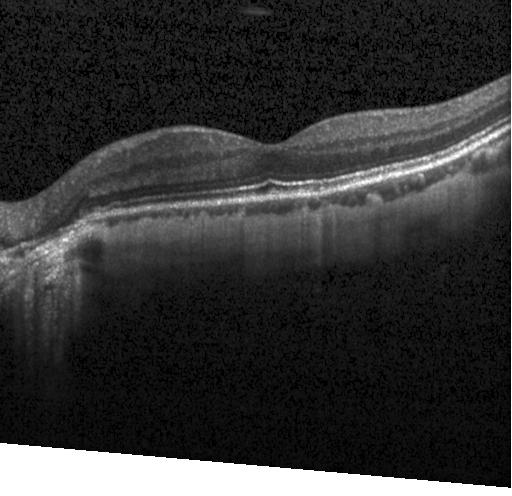 Impression: no choroidal neovascularization, no diabetic macular edema, and no drusen.